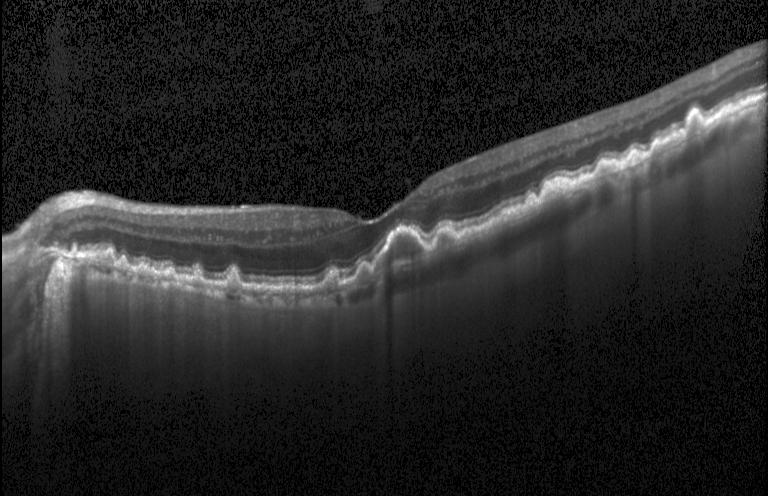
Retinal OCT cross-section showing multiple drusen.